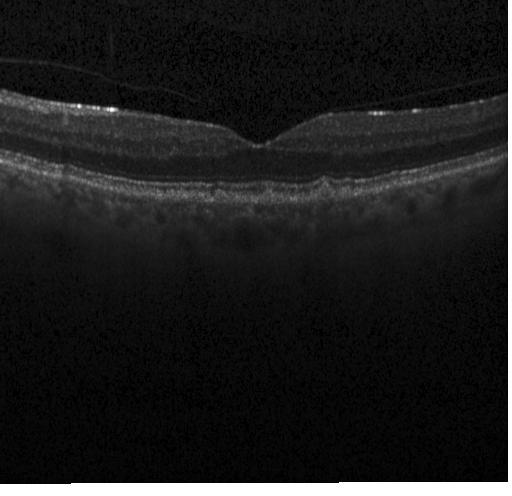 OCT B-scan showing drusen.